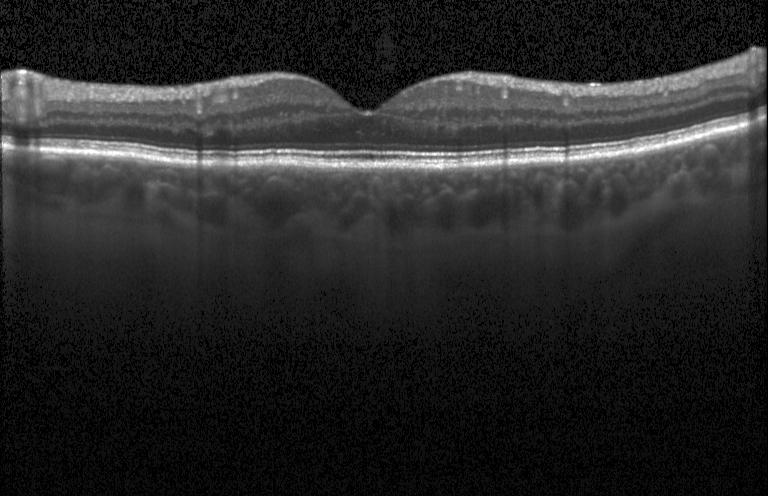
Through the macula, OCT B-scan.
Finding: no choroidal neovascularization, no diabetic macular edema, and no drusen.